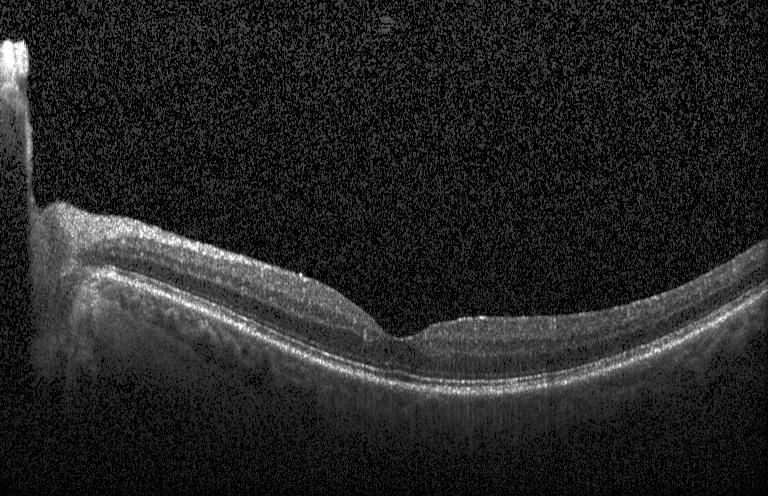
OCT B-scan. Fovea-centered. The scan shows neither CNV, DME, nor drusen.